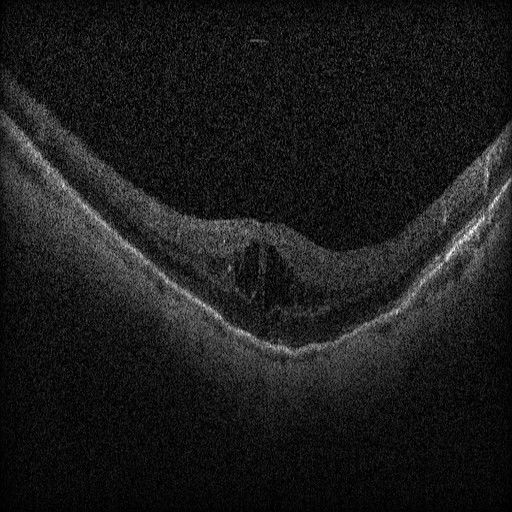
Retinal OCT cross-section showing diabetic macular edema.